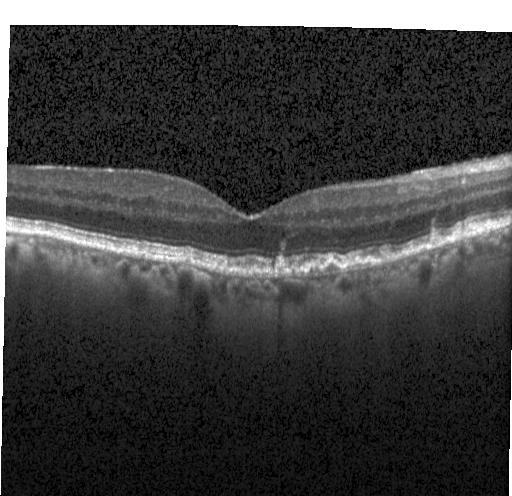

Horizontal scan through the fovea, OCT line scan, Heidelberg Spectralis, SD-OCT
OCT finding: sub-RPE drusenoid deposits.